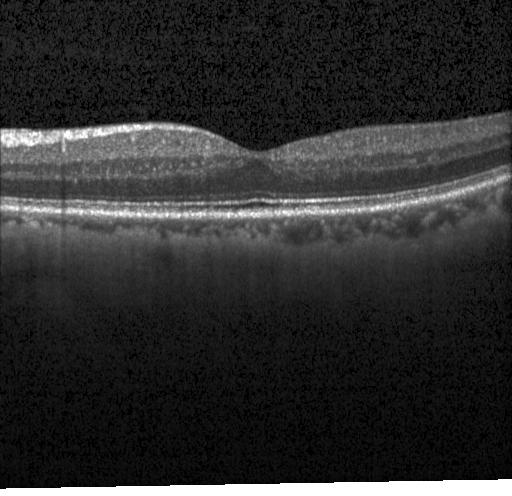

Dx: neither choroidal neovascularization, diabetic macular edema, nor drusen.